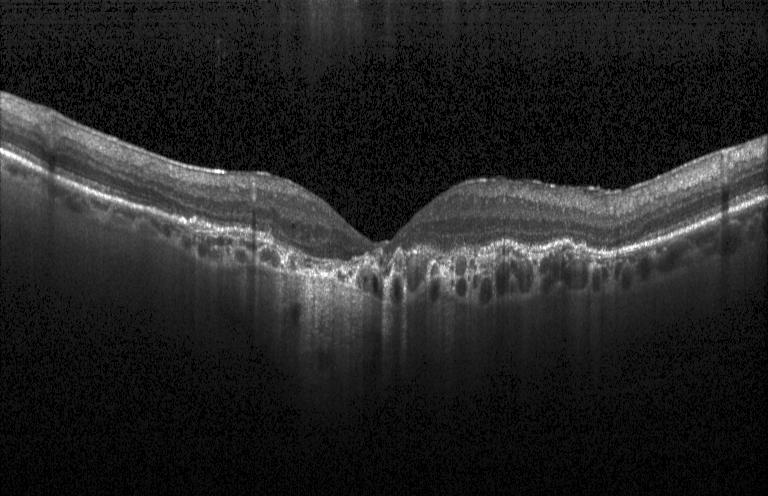

Retinal OCT cross-section. Heidelberg Spectralis. Horizontal scan through the fovea. SD-OCT
Impression: choroidal neovascularization (CNV).